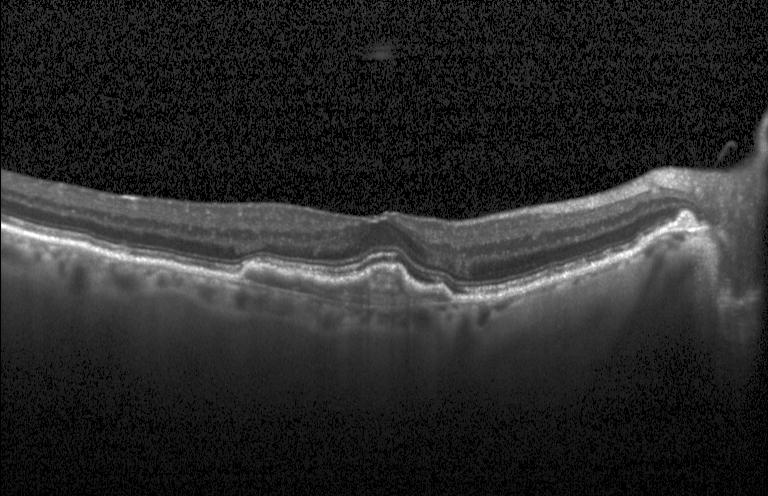

A choroidal neovascular membrane.